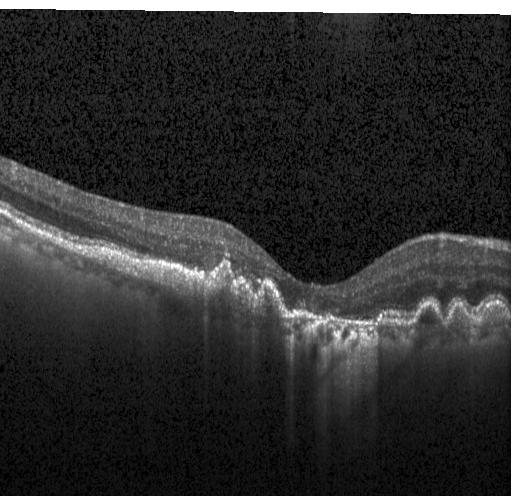 Heidelberg Spectralis, retinal OCT cross-section, spectral-domain OCT.
Assessment: choroidal neovascularization.